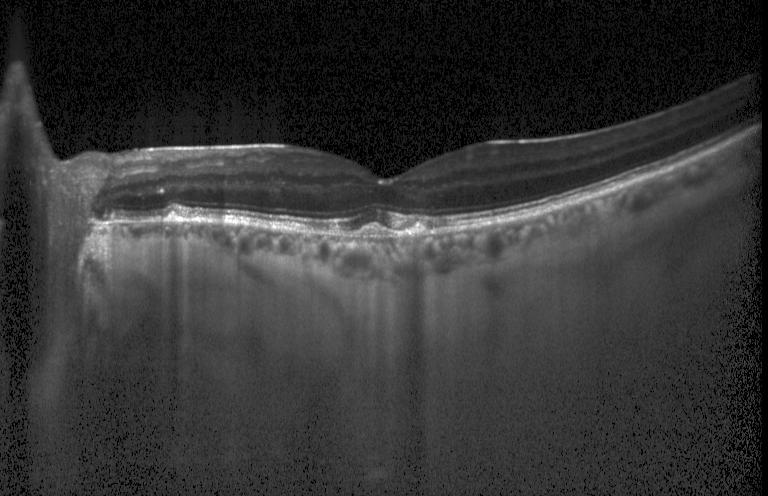 Optical coherence tomography B-scan · through the macula.
Impression: CNV.